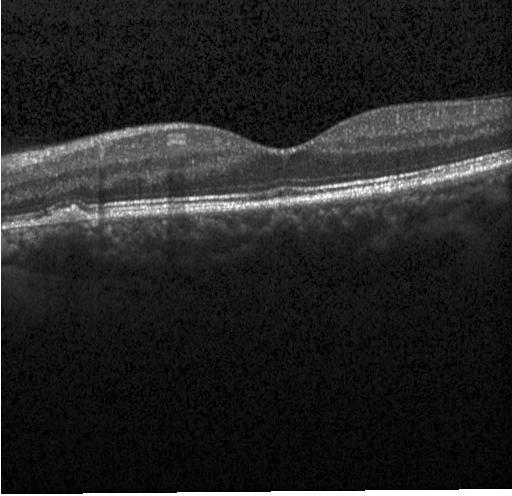

Heidelberg Spectralis OCT system, optical coherence tomography scan — Impression: sub-RPE drusenoid deposits.